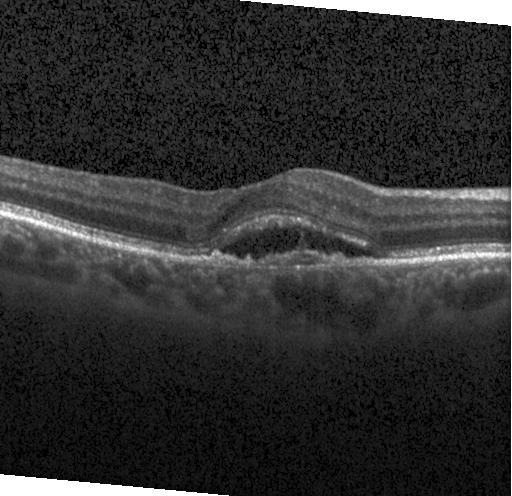
OCT B-scan.
Impression: CNV.